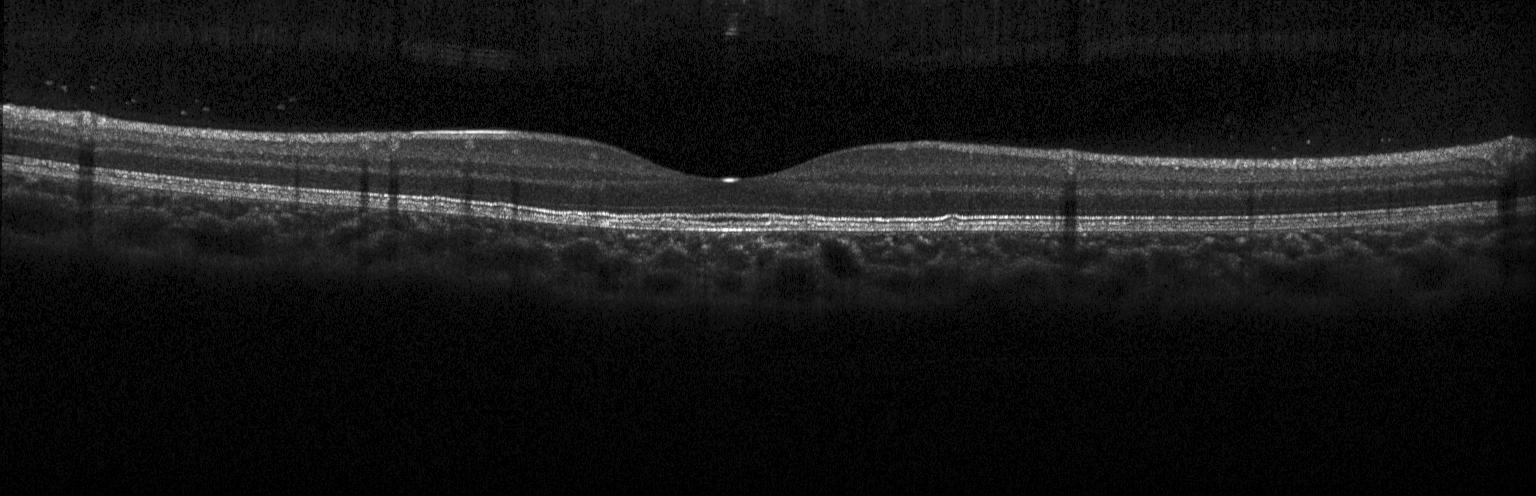
Optical coherence tomography scan, horizontal scan through the fovea, SD-OCT. Diagnosis: no evidence of CNV, DME, or drusen.